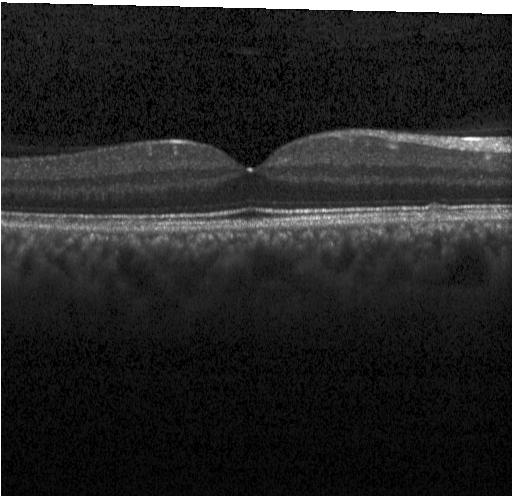
Optical coherence tomography scan
Finding: neither choroidal neovascularization, diabetic macular edema, nor drusen.